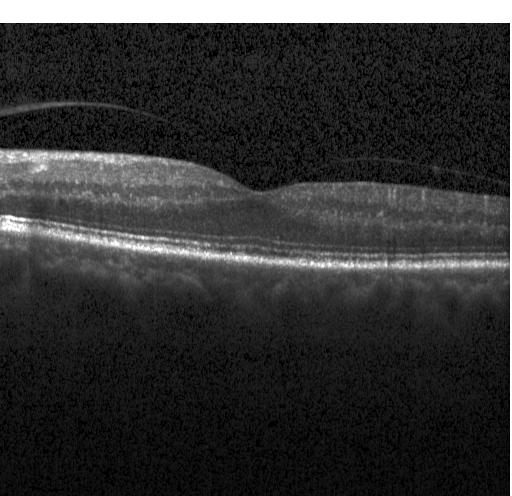

Instrument: Heidelberg Spectralis. Centered on the fovea. Optical coherence tomography B-scan. The scan shows no evidence of CNV, DME, or drusen.